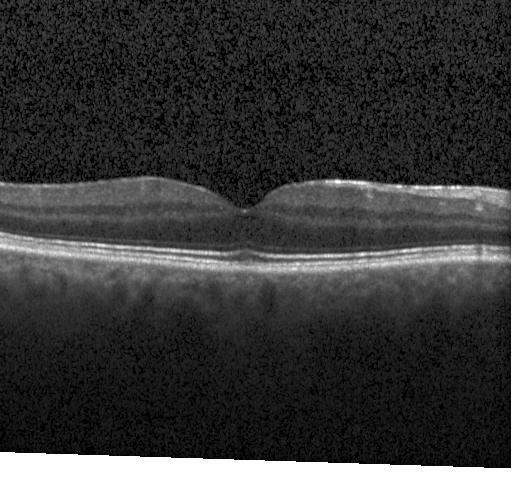
Finding: no choroidal neovascularization, diabetic macular edema, or drusen.